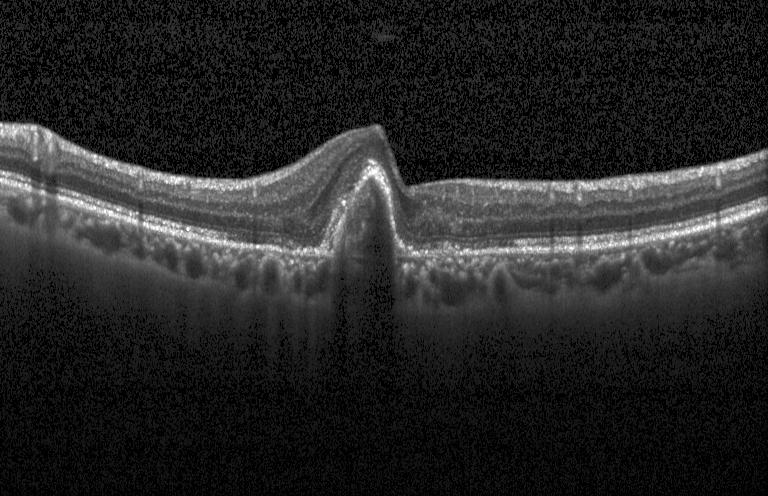
Optical coherence tomography B-scan — Diagnosis: choroidal neovascularization (CNV).